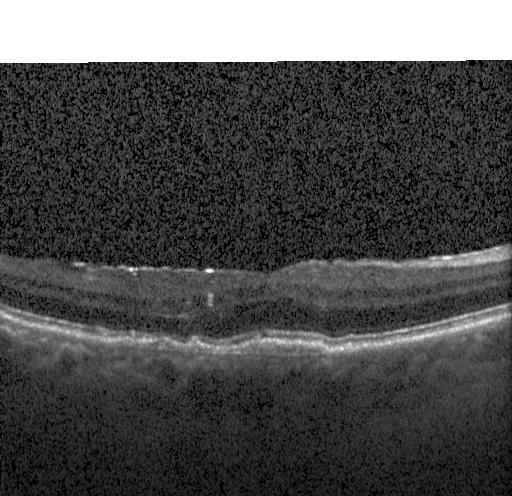

Heidelberg Spectralis. OCT line scan. Through the macula. Macular OCT: choroidal neovascularization.